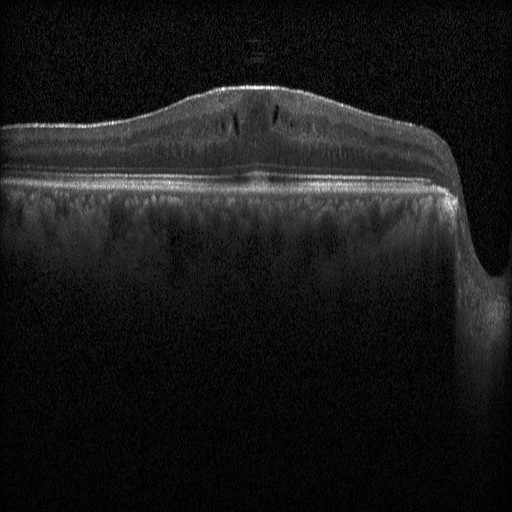 OCT line scan — Macular OCT: diabetic macular edema.